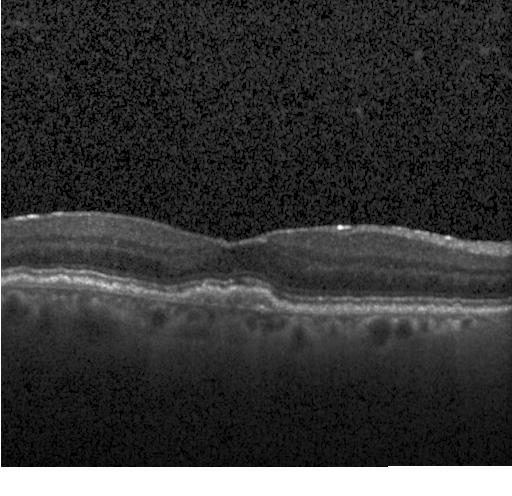
This B-scan demonstrates a choroidal neovascular membrane.